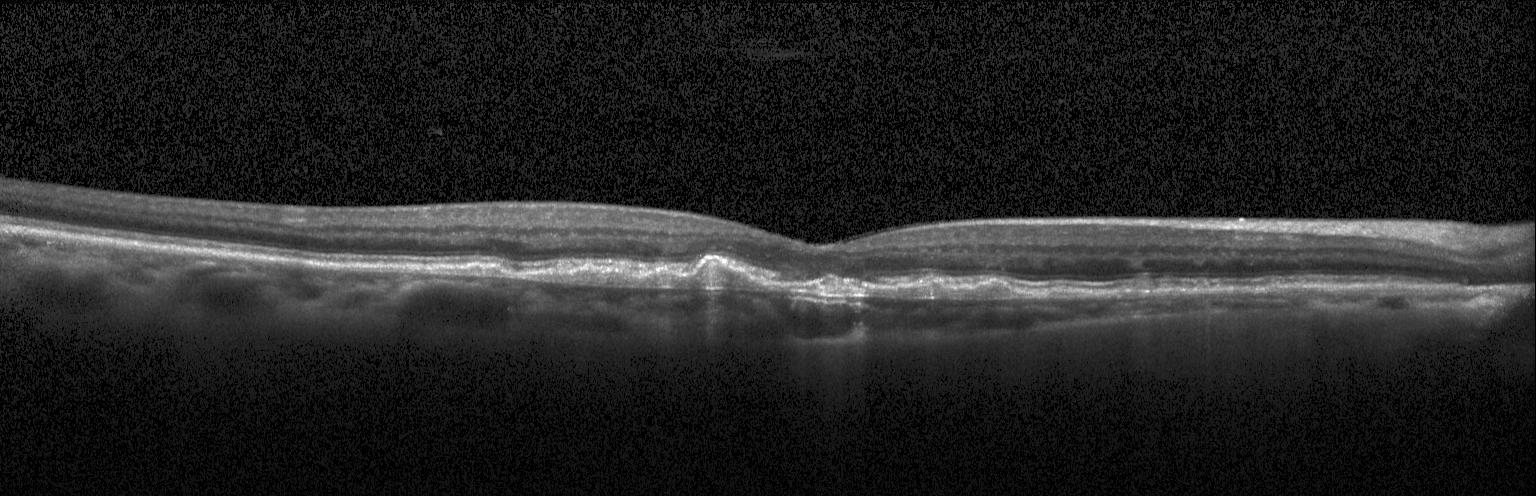
Retinal OCT cross-section showing a choroidal neovascular membrane.